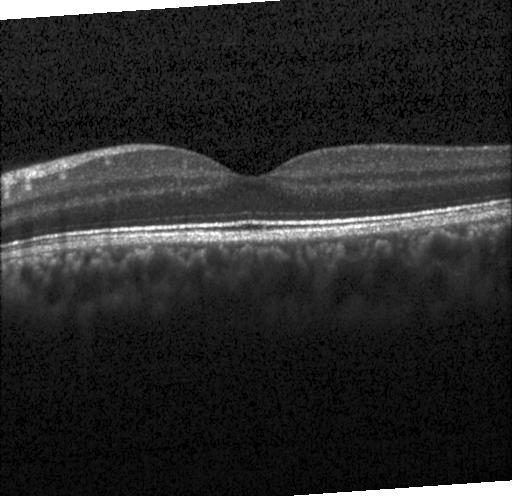
This B-scan demonstrates no choroidal neovascularization, diabetic macular edema, or drusen.